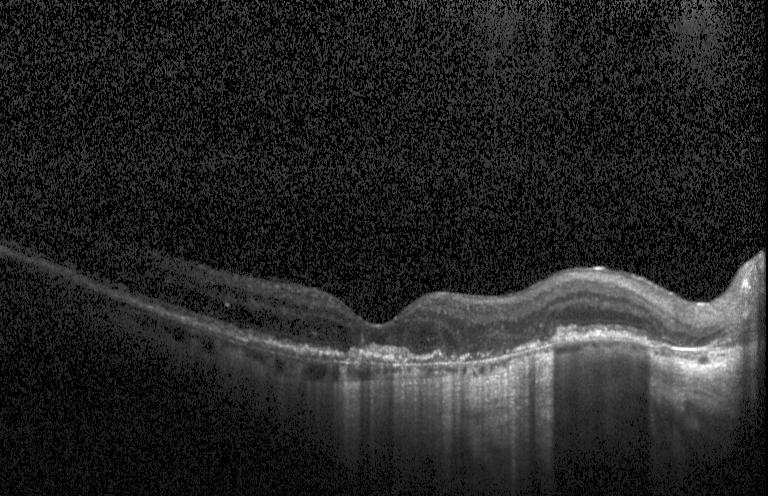

Centered on the fovea · SD-OCT · Heidelberg Spectralis OCT system · OCT line scan — CNV.